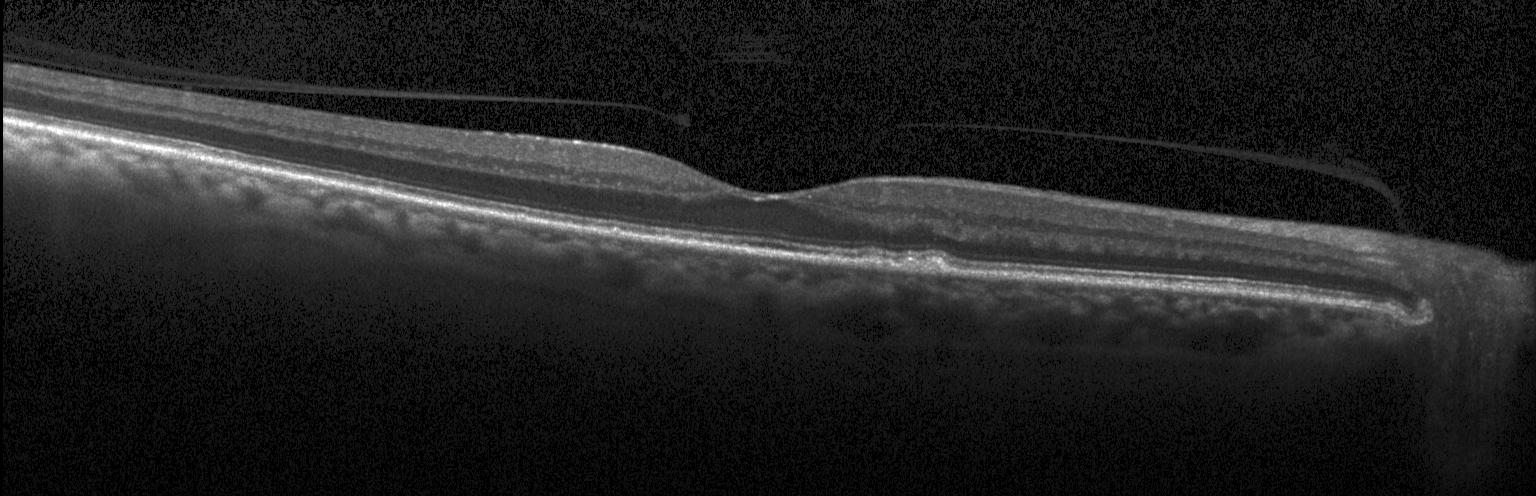

Multiple drusen.